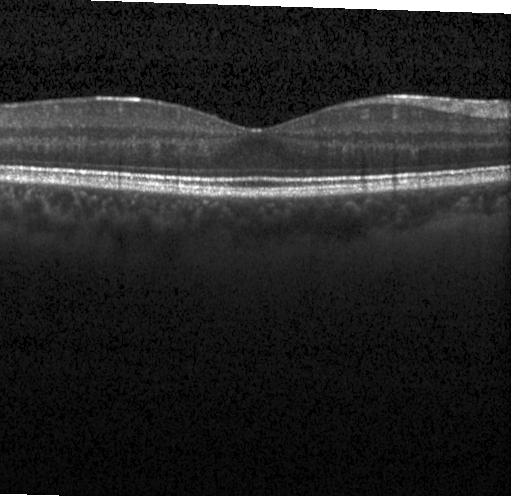
OCT B-scan showing no CNV, DME, or drusen.